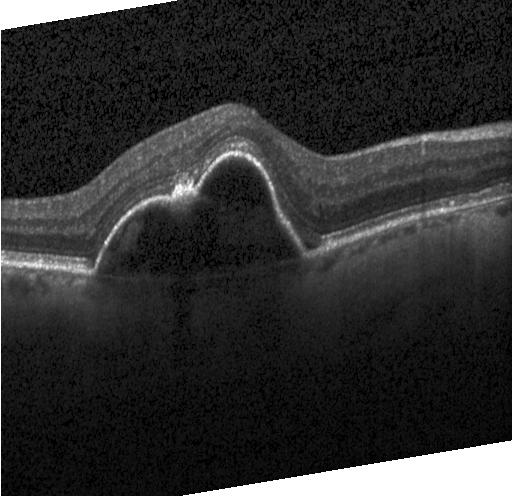

OCT B-scan. Heidelberg Spectralis. SD-OCT
Finding: a choroidal neovascular membrane.